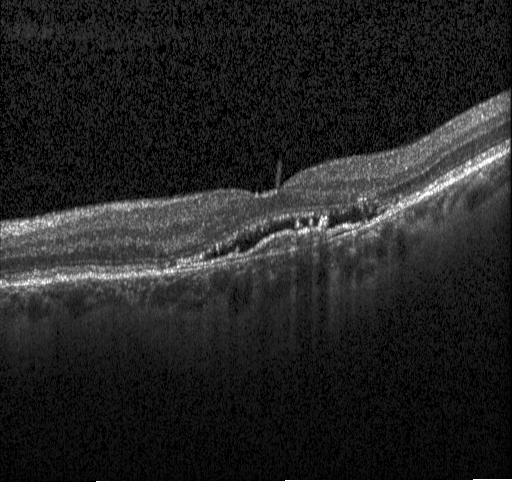 Heidelberg Spectralis OCT system; retinal OCT B-scan; macular scan. Finding: a choroidal neovascular membrane.